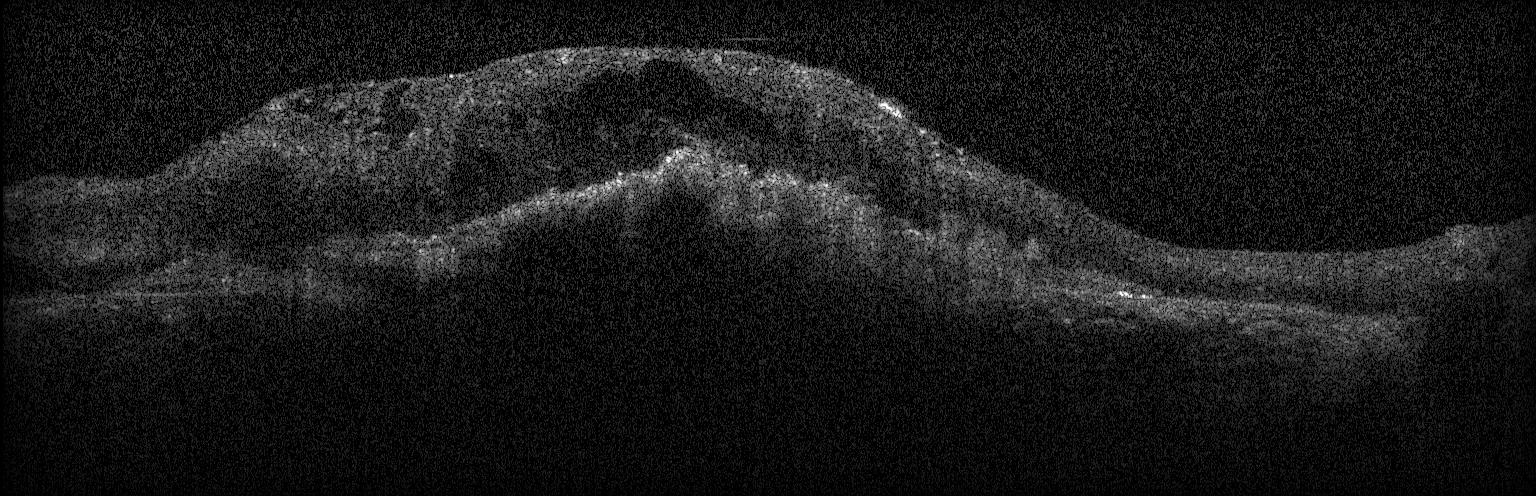

Optical coherence tomography scan, centered on the fovea. This B-scan demonstrates a choroidal neovascular membrane.